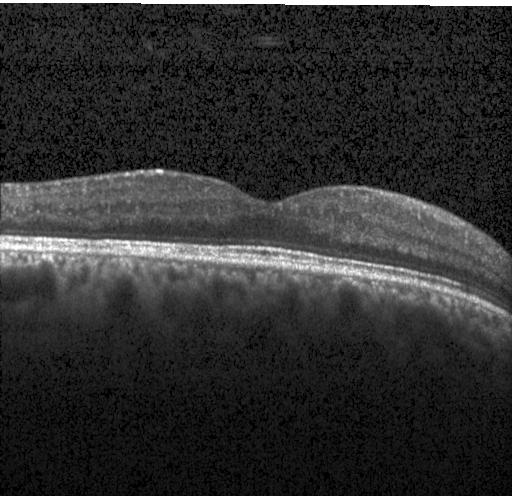

The scan shows no CNV, DME, or drusen.